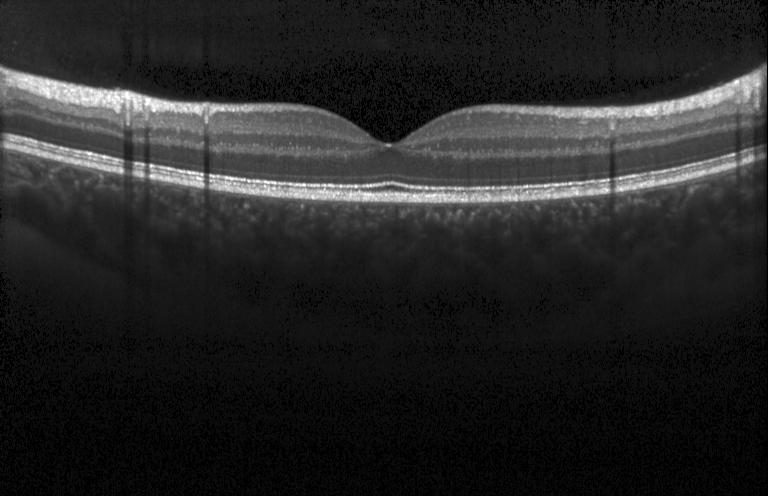 OCT B-scan showing no choroidal neovascularization, no diabetic macular edema, and no drusen.